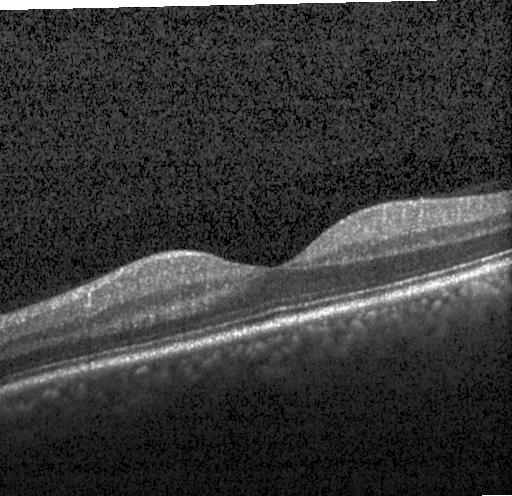 Retinal OCT cross-section · spectral-domain OCT — This B-scan demonstrates neither choroidal neovascularization, diabetic macular edema, nor drusen.